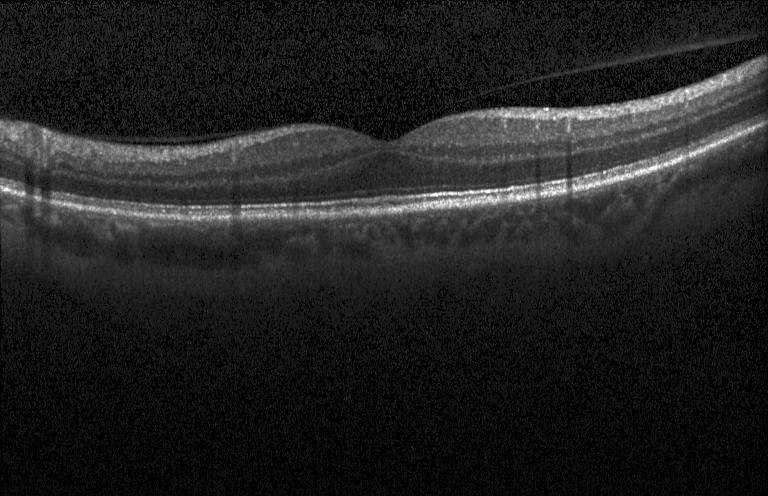 Spectral-domain OCT · retinal OCT cross-section · acquired on a Heidelberg Spectralis · centered on the fovea.
Macular OCT: no evidence of CNV, DME, or drusen.